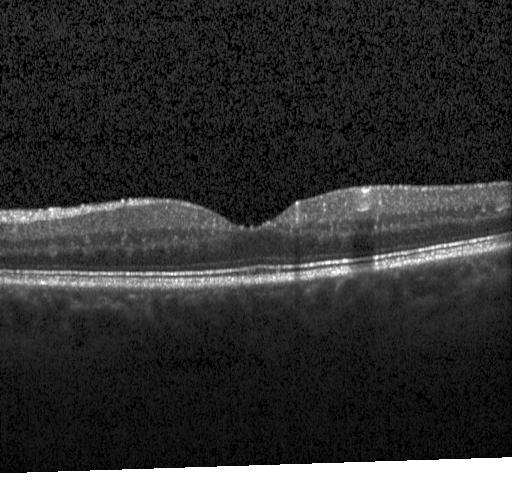

OCT finding: no choroidal neovascularization, diabetic macular edema, or drusen.